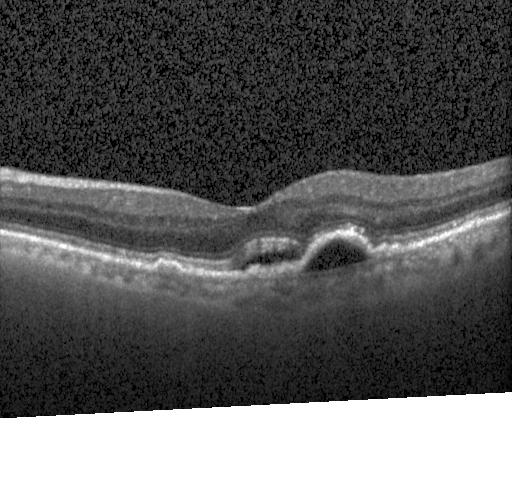 OCT B-scan — Impression: a choroidal neovascular membrane.